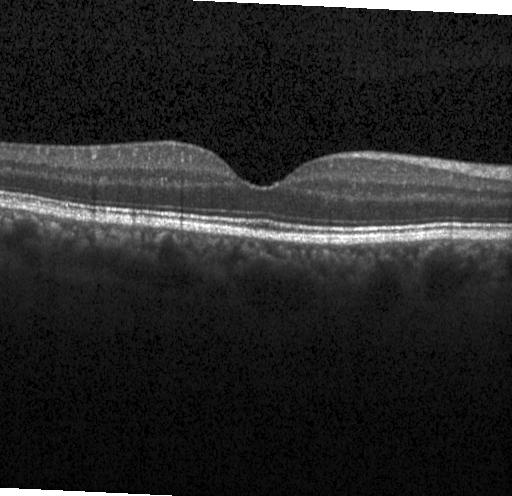

Impression: no CNV, DME, or drusen.